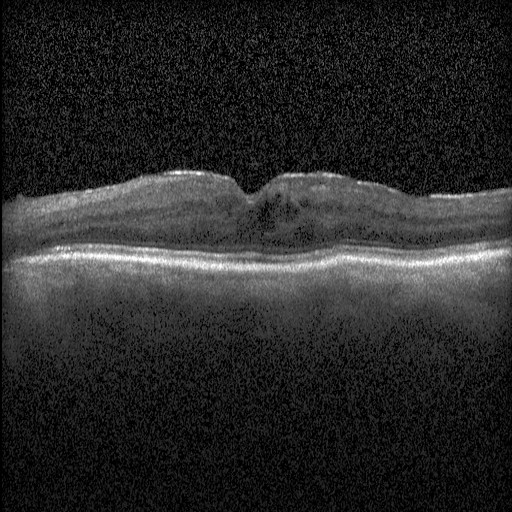

Retinal OCT cross-section · instrument: Heidelberg Spectralis · centered on the fovea — Macular OCT: diabetic macular edema (DME).